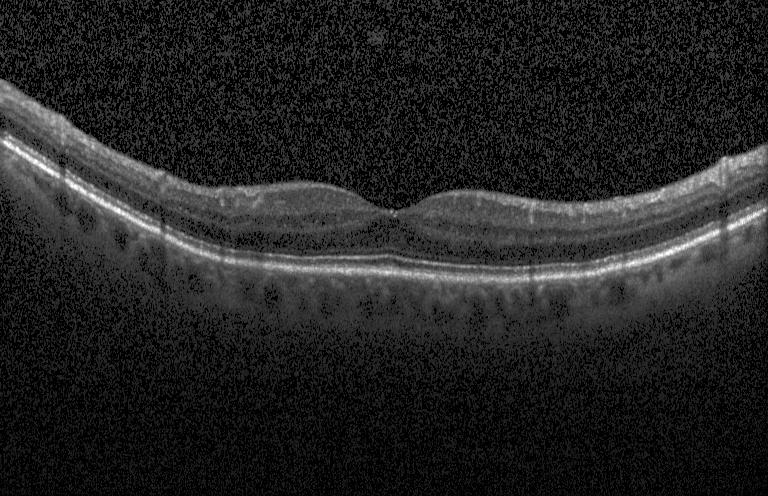 Diagnosis: neither choroidal neovascularization, diabetic macular edema, nor drusen.